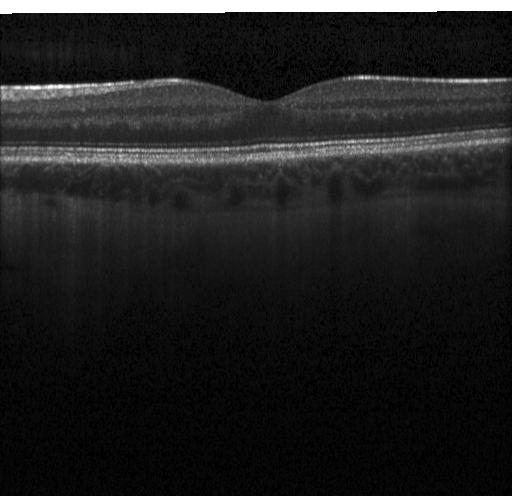
Retinal OCT cross-section. Macular scan
Diagnosis: neither choroidal neovascularization, diabetic macular edema, nor drusen.